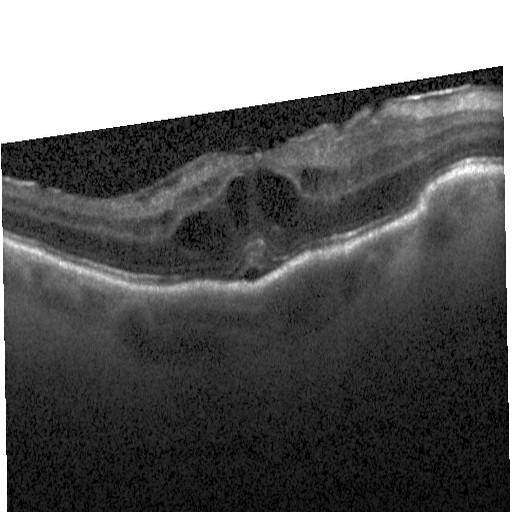

Centered on the fovea, OCT line scan
Dx: diabetic macular edema.